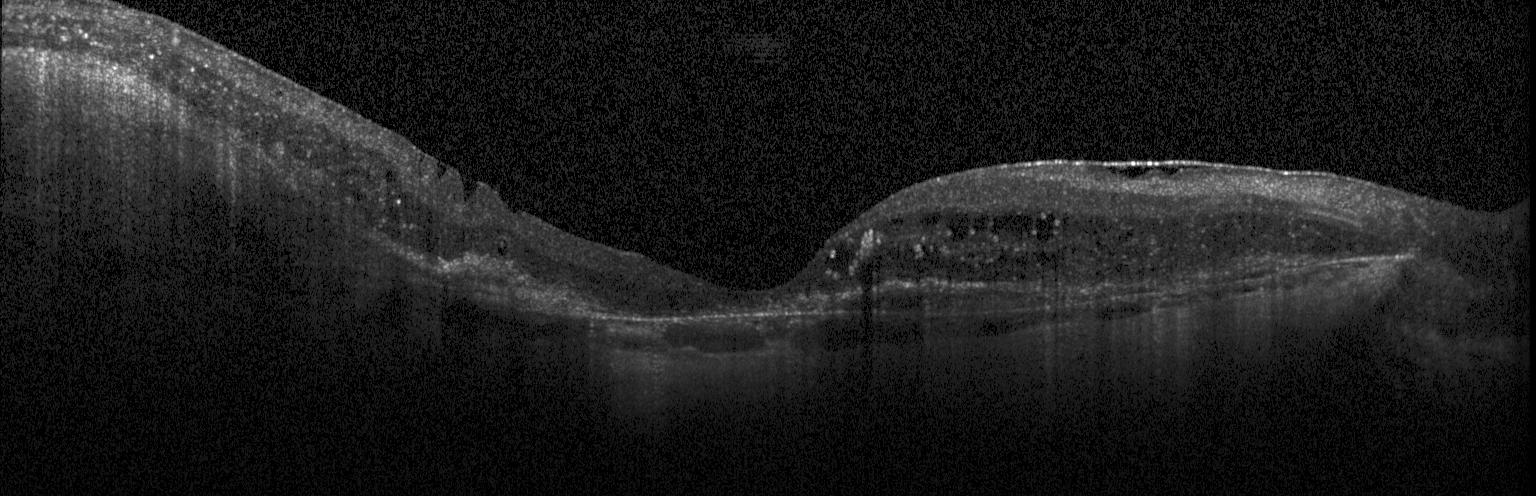
Optical coherence tomography scan.
Choroidal neovascularization (CNV).